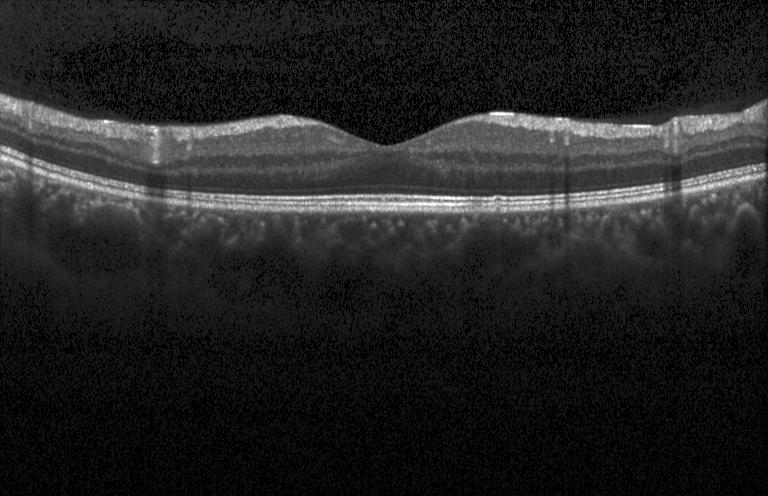

Assessment: no choroidal neovascularization, diabetic macular edema, or drusen.